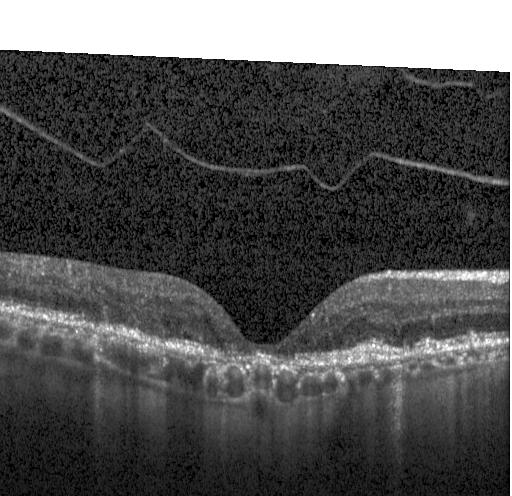 Macular scan · optical coherence tomography B-scan
Diagnosis: a choroidal neovascular membrane.